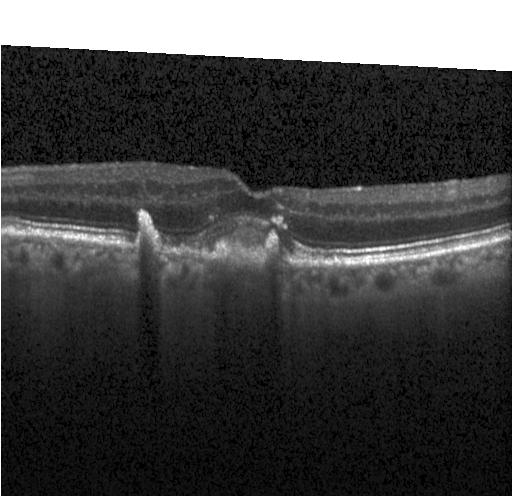 Finding: a choroidal neovascular membrane.